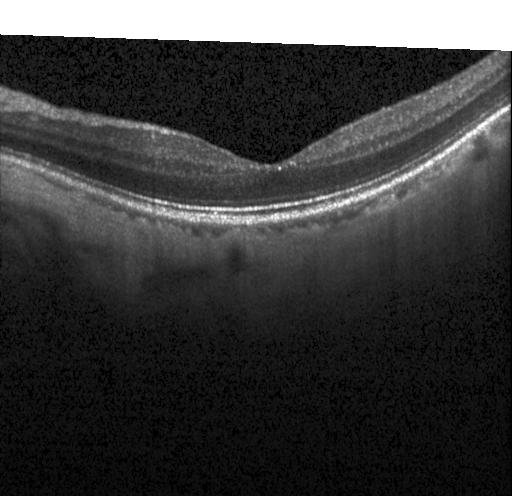
Acquired on a Heidelberg Spectralis, OCT line scan — Assessment: no choroidal neovascularization, no diabetic macular edema, and no drusen.